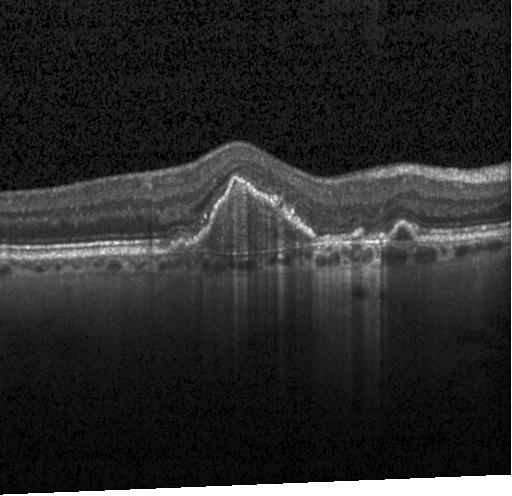
Optical coherence tomography scan.
Diagnosis: CNV.